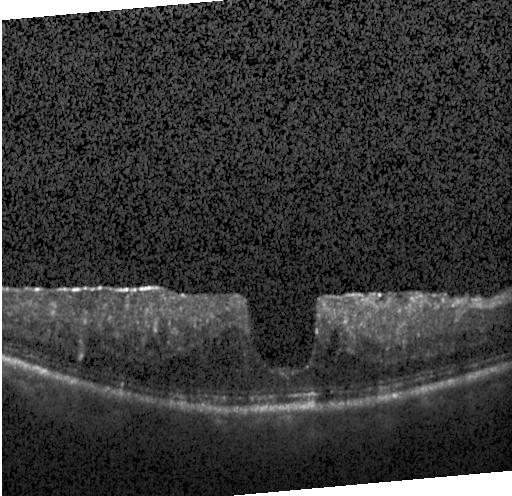

Dx: DME.